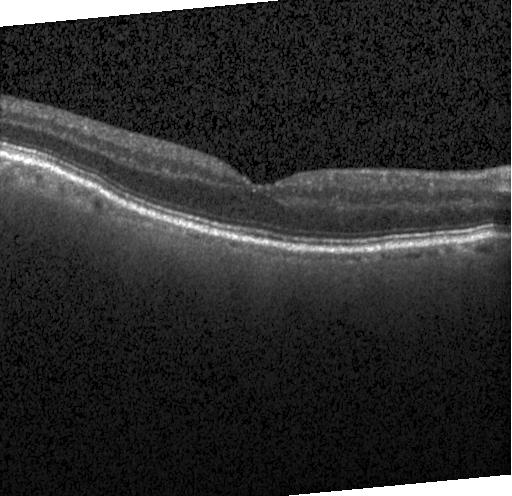
Macular OCT: neither choroidal neovascularization, diabetic macular edema, nor drusen.